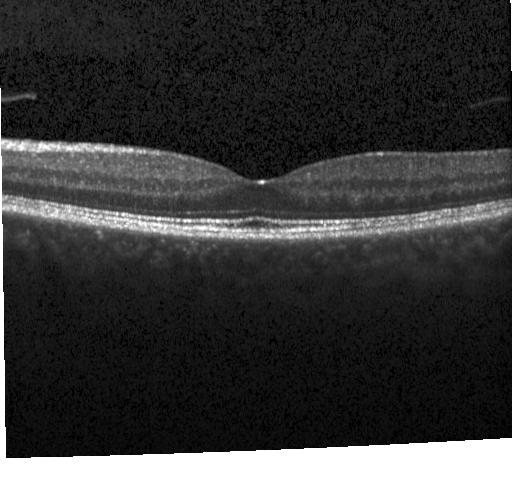 Spectral-domain OCT; optical coherence tomography scan; centered on the fovea
Impression: no choroidal neovascularization, no diabetic macular edema, and no drusen.